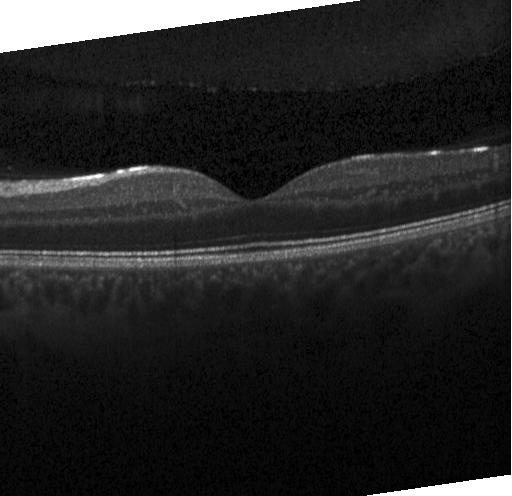 No CNV, DME, or drusen.